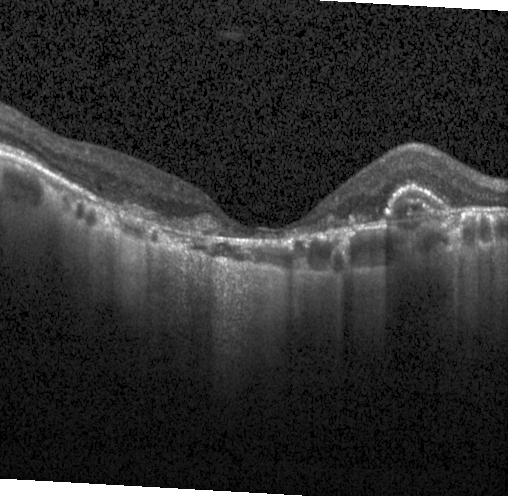
OCT B-scan showing choroidal neovascularization (CNV).